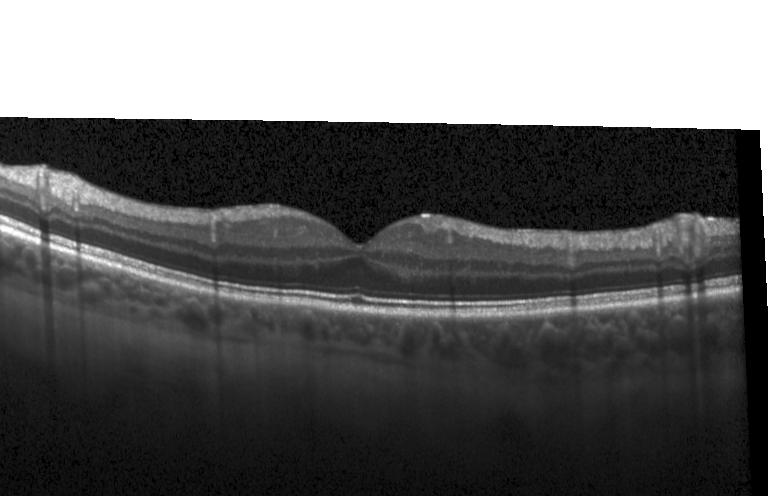

OCT line scan; centered on the fovea
Assessment: no choroidal neovascularization, diabetic macular edema, or drusen.